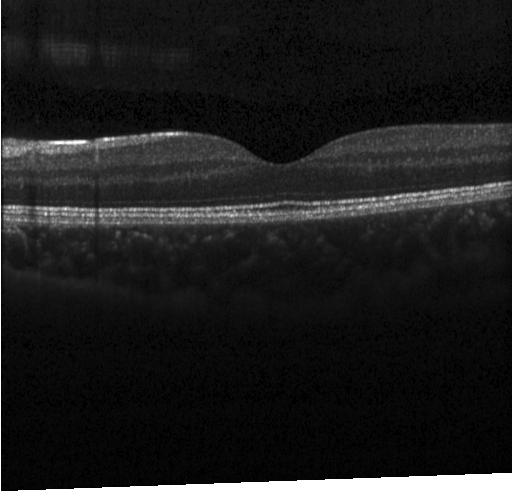 OCT B-scan
Diagnosis: neither choroidal neovascularization, diabetic macular edema, nor drusen.